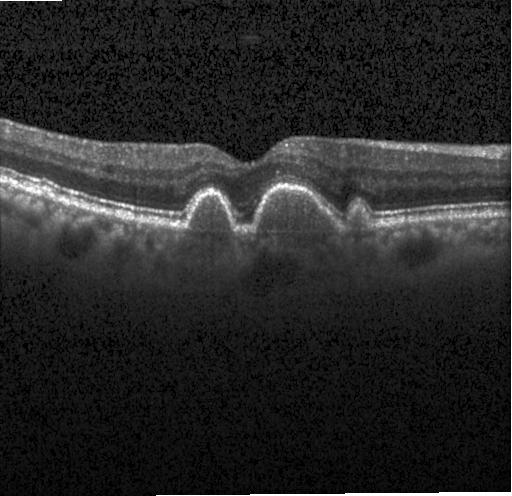

Spectral-domain OCT B-scan: sub-RPE drusenoid deposits.